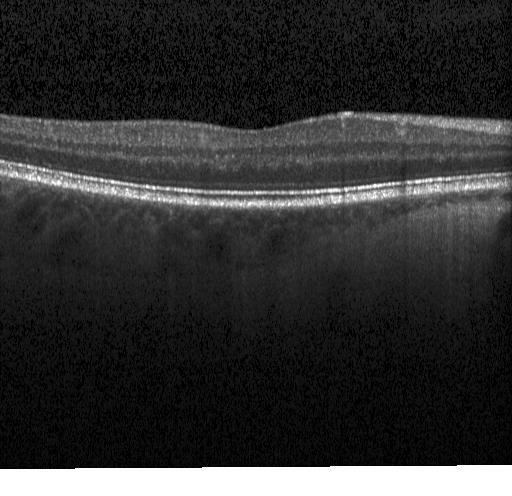

SD-OCT; retinal OCT B-scan; centered on the fovea
Diagnosis: no choroidal neovascularization, diabetic macular edema, or drusen.